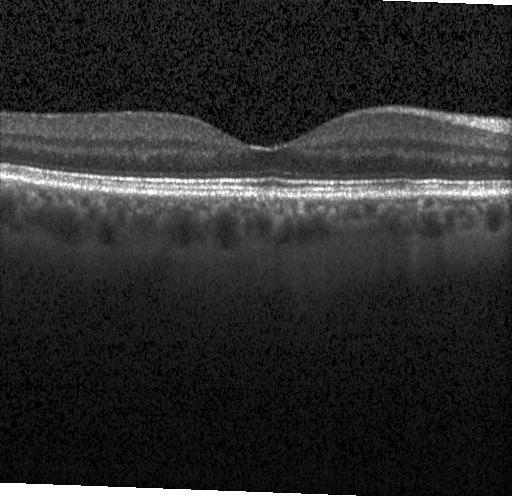

Optical coherence tomography B-scan, Heidelberg Spectralis, horizontal scan through the fovea.
Finding: neither choroidal neovascularization, diabetic macular edema, nor drusen.